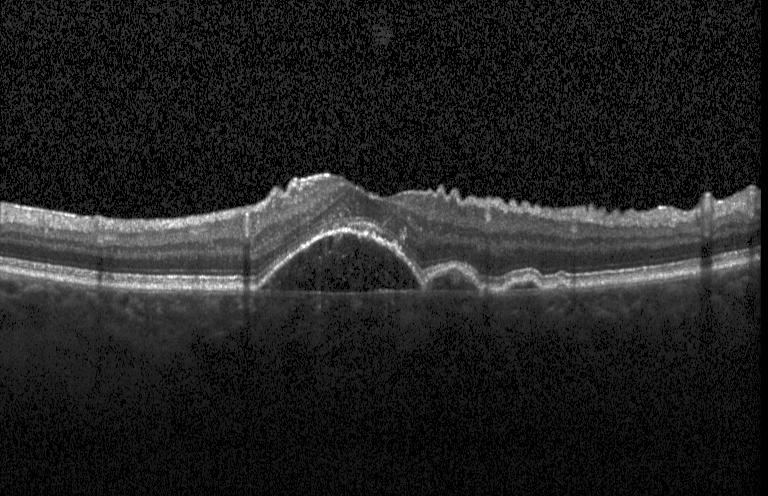 Diagnosis: choroidal neovascularization.